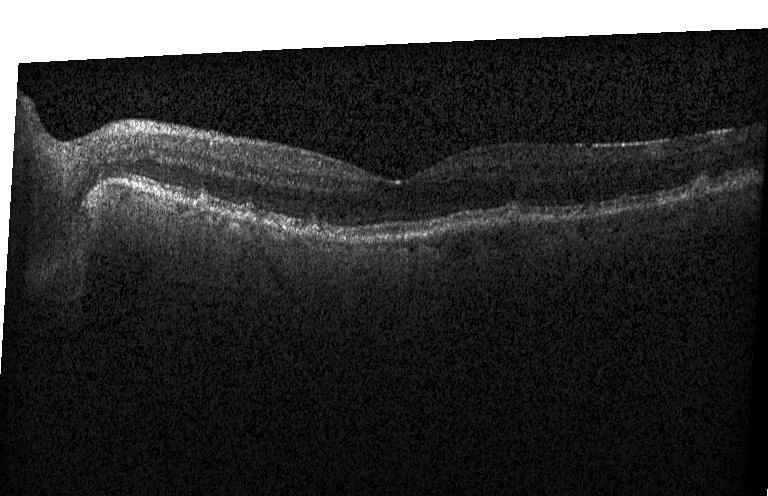

Instrument: Heidelberg Spectralis, fovea-centered, optical coherence tomography B-scan — Assessment: drusen.